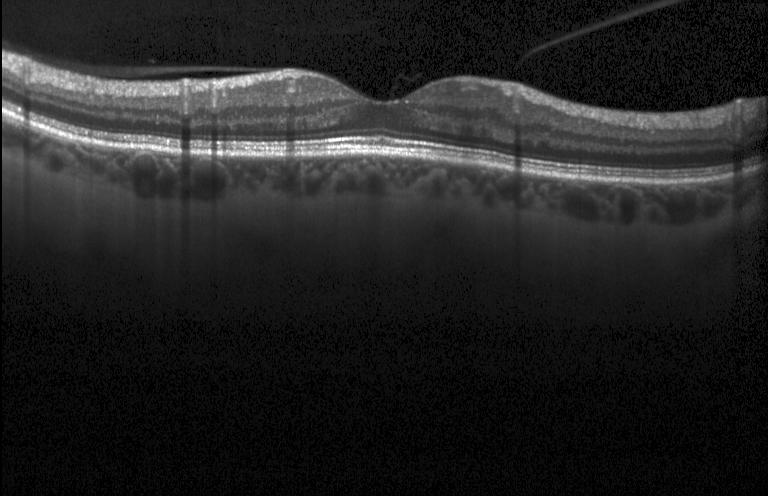
Spectral-domain OCT, optical coherence tomography B-scan, instrument: Heidelberg Spectralis, macular scan. Finding: neither choroidal neovascularization, diabetic macular edema, nor drusen.